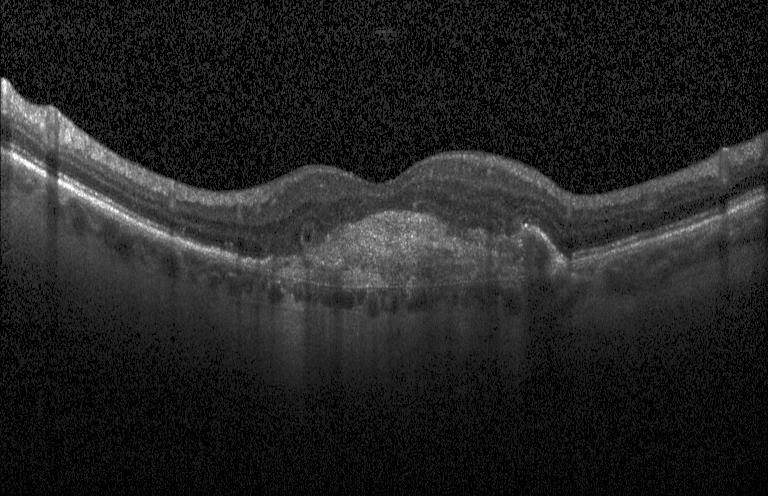
Impression: a choroidal neovascular membrane.